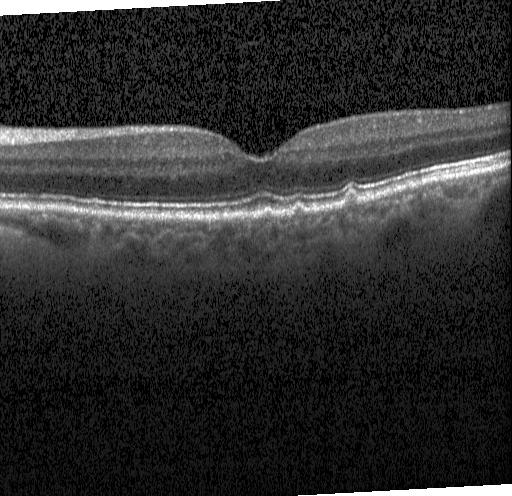
Retinal OCT cross-section. Diagnosis: sub-RPE drusenoid deposits.